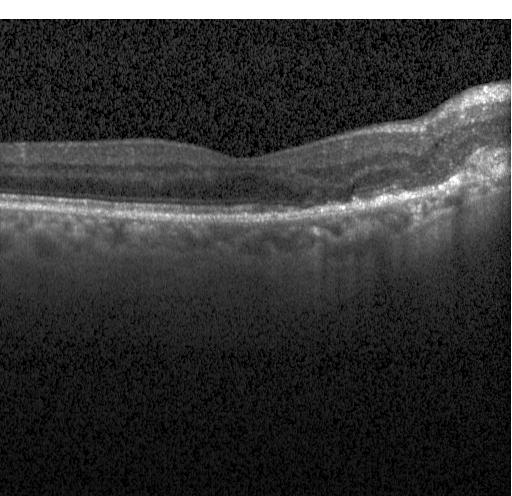

OCT B-scan showing a choroidal neovascular membrane.